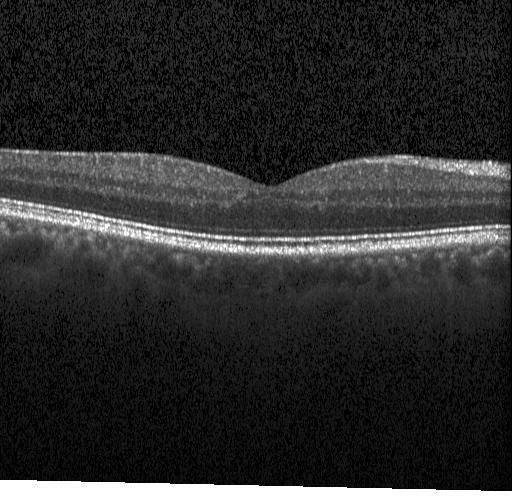

Macular OCT demonstrating no choroidal neovascularization, diabetic macular edema, or drusen.